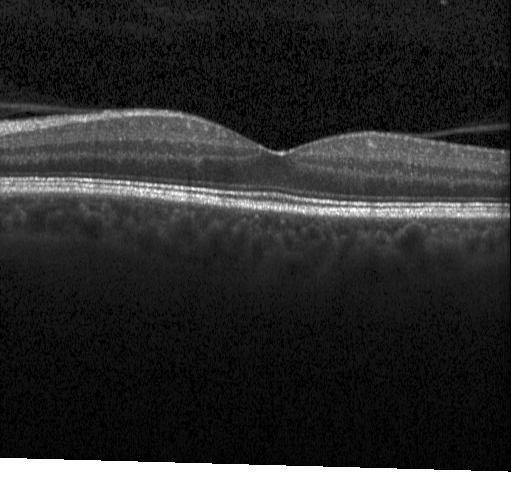

Impression: no CNV, DME, or drusen.